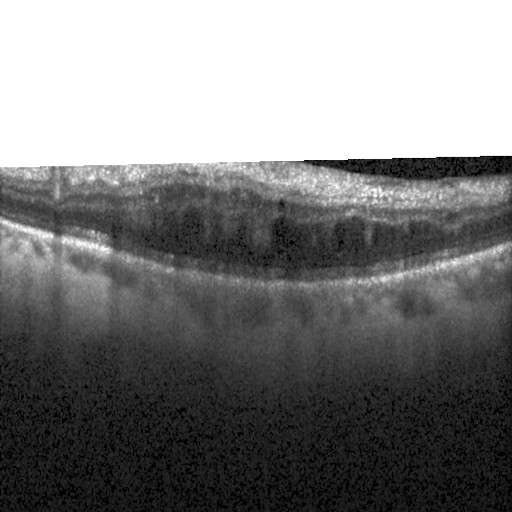

Through the macula; retinal OCT B-scan; SD-OCT.
Diagnosis: diabetic macular edema.